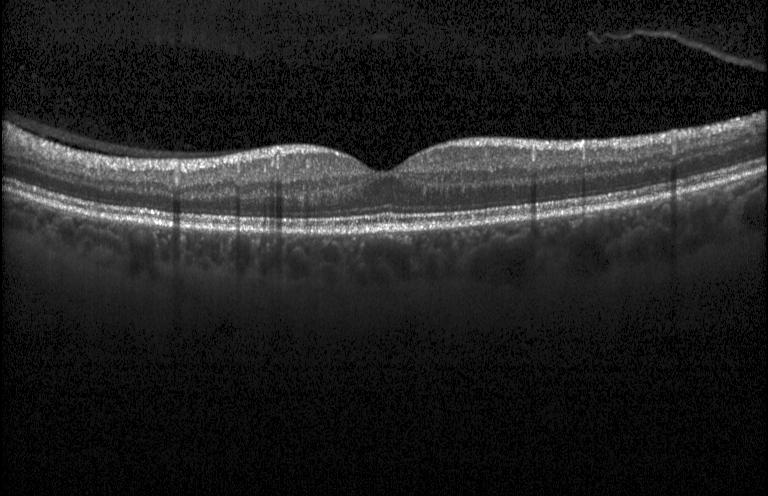

OCT B-scan · spectral-domain optical coherence tomography. Diagnosis: no choroidal neovascularization, no diabetic macular edema, and no drusen.